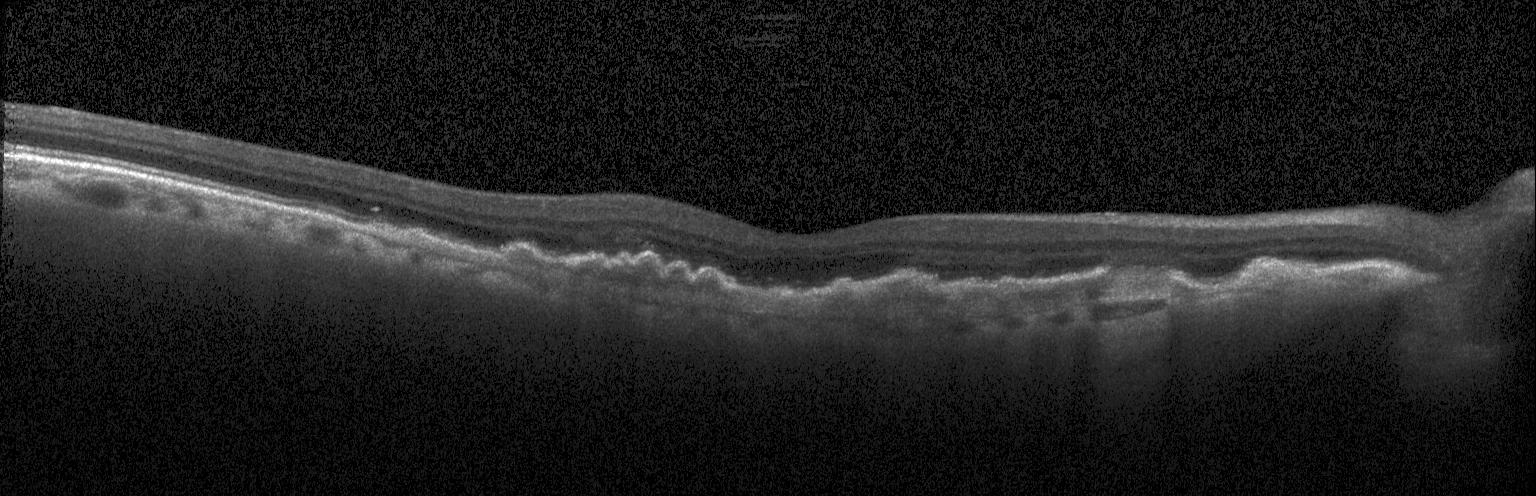
Optical coherence tomography B-scan. Centered on the fovea. Acquired on a Heidelberg Spectralis
Dx: a choroidal neovascular membrane.